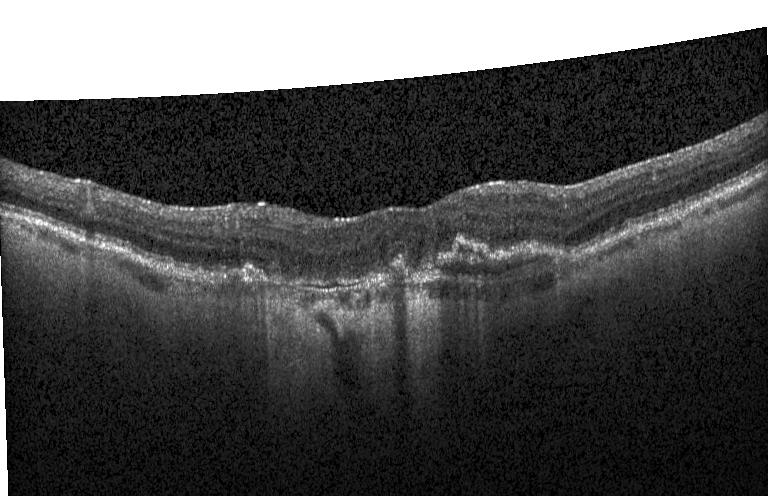 Optical coherence tomography B-scan · Heidelberg Spectralis OCT system · fovea-centered.
This B-scan demonstrates CNV.